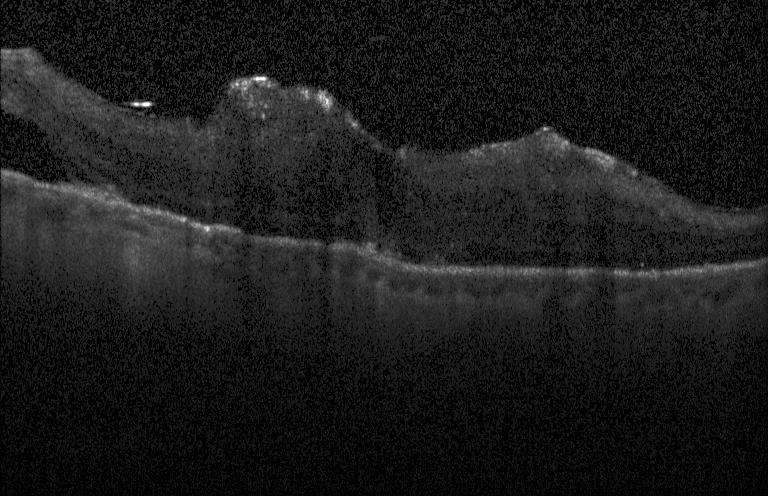

Macular scan. Optical coherence tomography B-scan.
Diagnosis: diabetic macular edema.